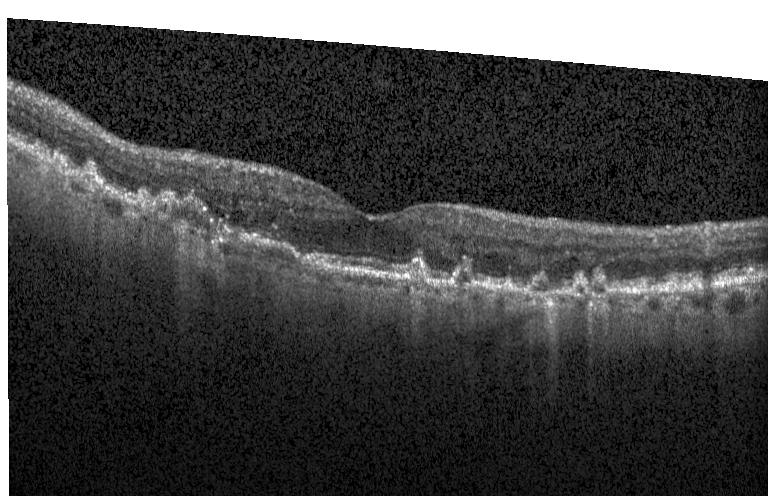
OCT B-scan; fovea-centered; SD-OCT
The scan shows choroidal neovascularization.